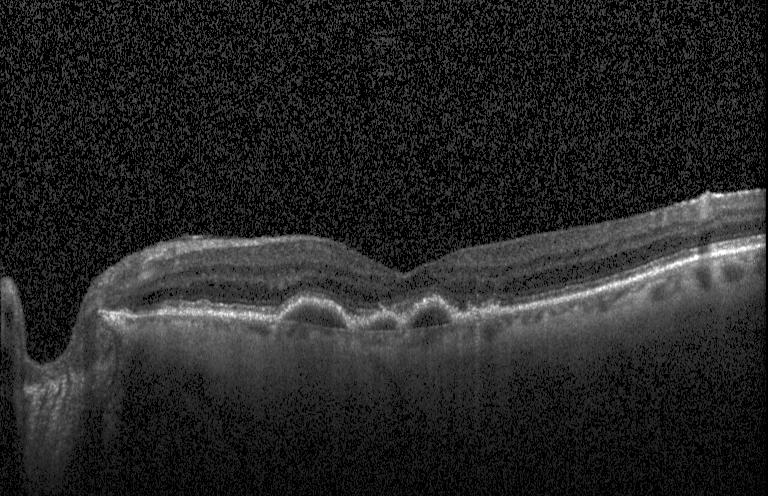
OCT finding: choroidal neovascularization.